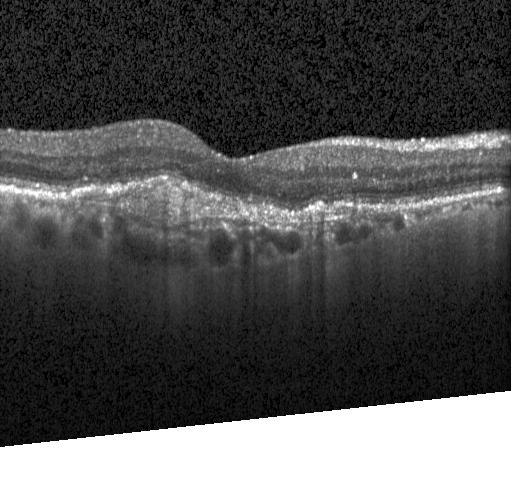

Dx: choroidal neovascularization (CNV).